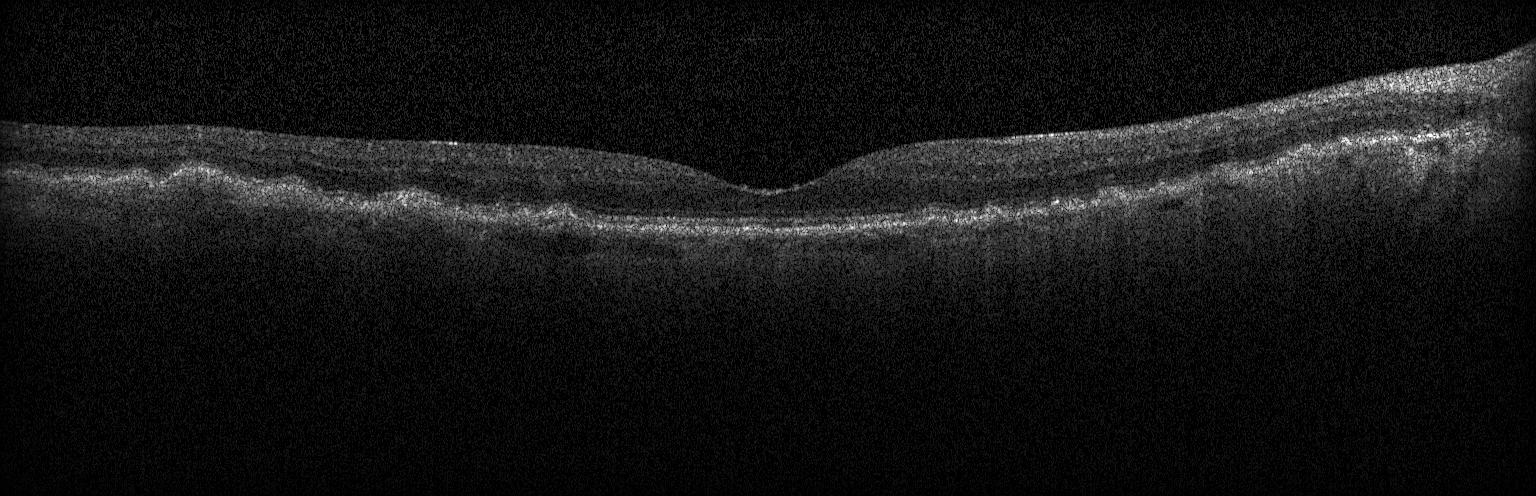 Retinal OCT cross-section showing drusen.